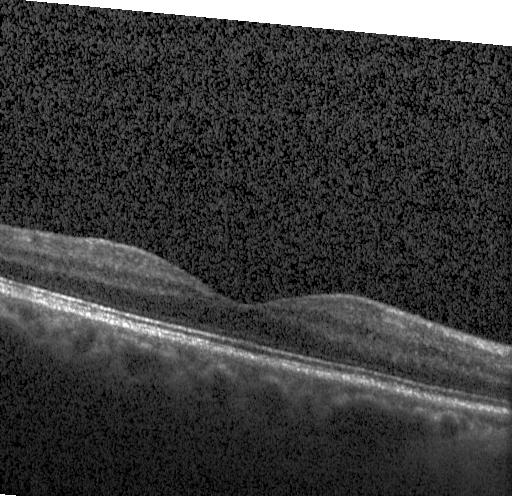
Acquired on a Heidelberg Spectralis; horizontal scan through the fovea; optical coherence tomography B-scan
No CNV, DME, or drusen.